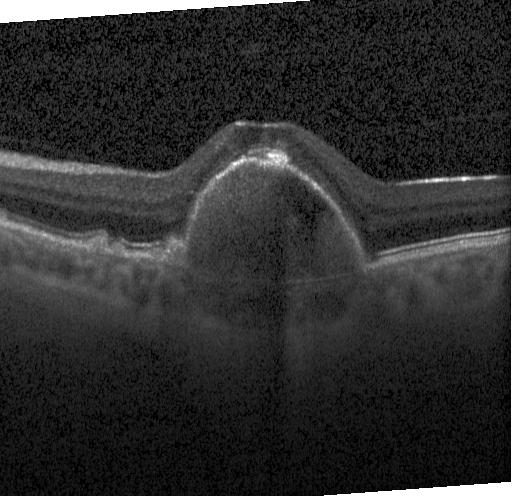
Diagnosis: choroidal neovascularization (CNV).